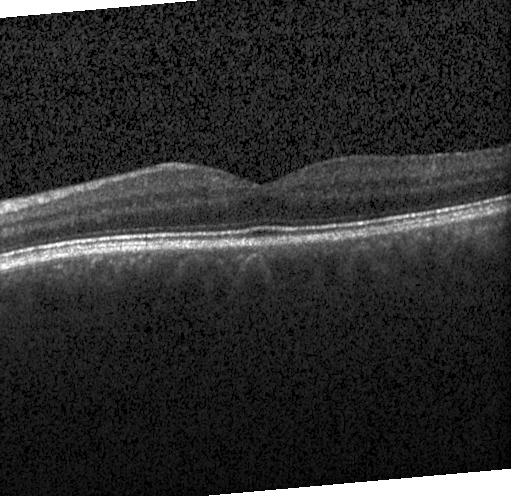

Macular scan. Instrument: Heidelberg Spectralis. SD-OCT. Optical coherence tomography B-scan.
OCT finding: no CNV, no DME, and no drusen.